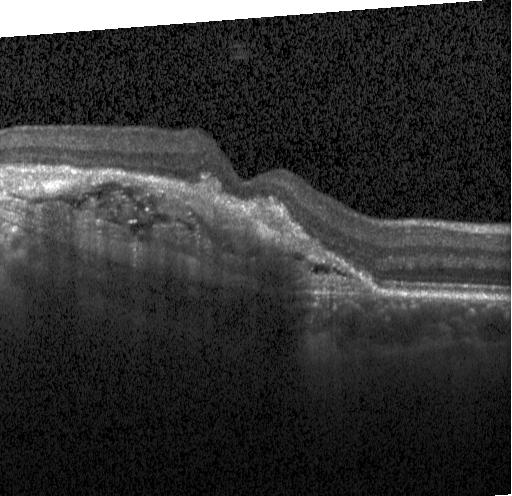 This B-scan demonstrates a choroidal neovascular membrane.